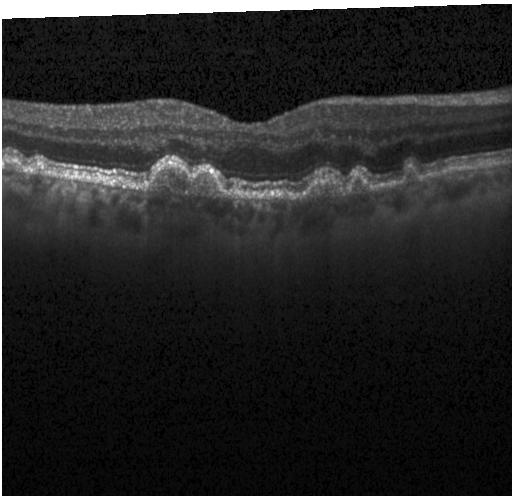
This B-scan demonstrates sub-RPE drusenoid deposits.